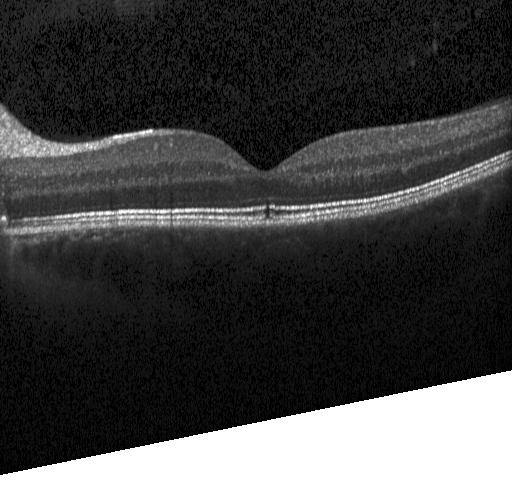

Macular OCT: neither CNV, DME, nor drusen.